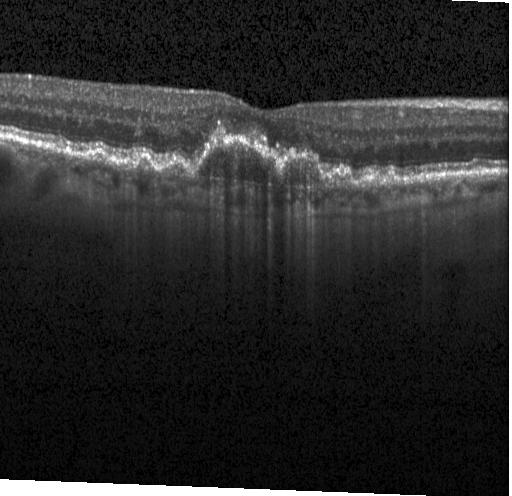 The scan shows a choroidal neovascular membrane.